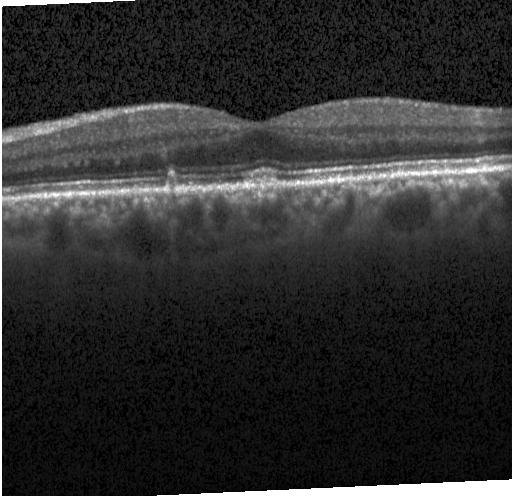 Horizontal scan through the fovea, spectral-domain OCT, OCT B-scan. Dx: multiple drusen.